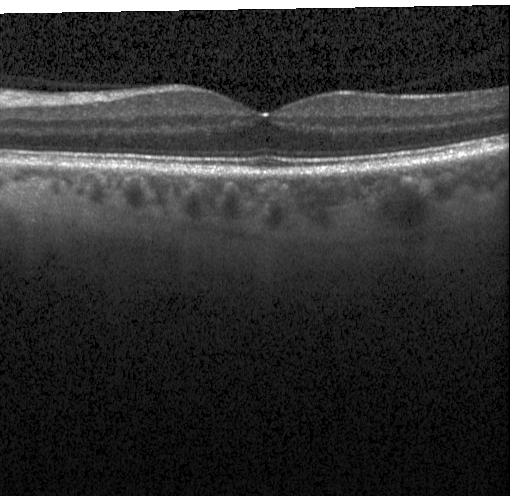 Impression: neither choroidal neovascularization, diabetic macular edema, nor drusen.